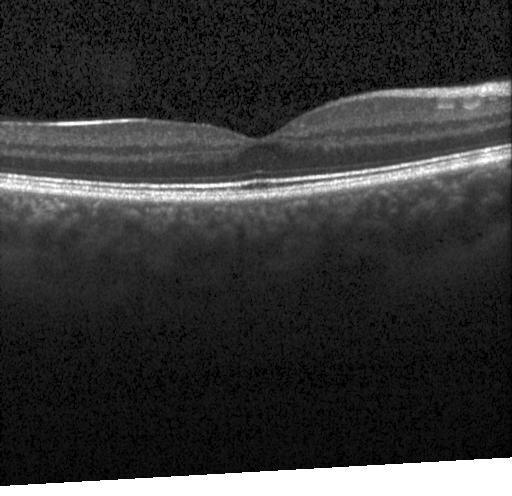 SD-OCT. Optical coherence tomography scan.
Finding: no CNV, no DME, and no drusen.